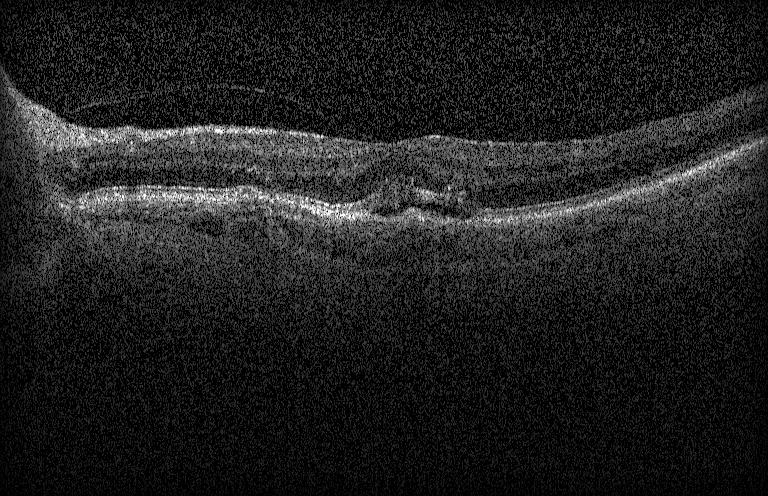

OCT finding: choroidal neovascularization.